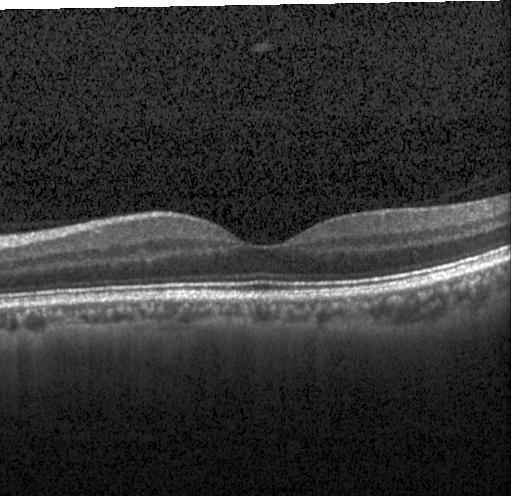
Heidelberg Spectralis · spectral-domain optical coherence tomography · macular scan · optical coherence tomography B-scan.
This B-scan demonstrates no choroidal neovascularization, no diabetic macular edema, and no drusen.